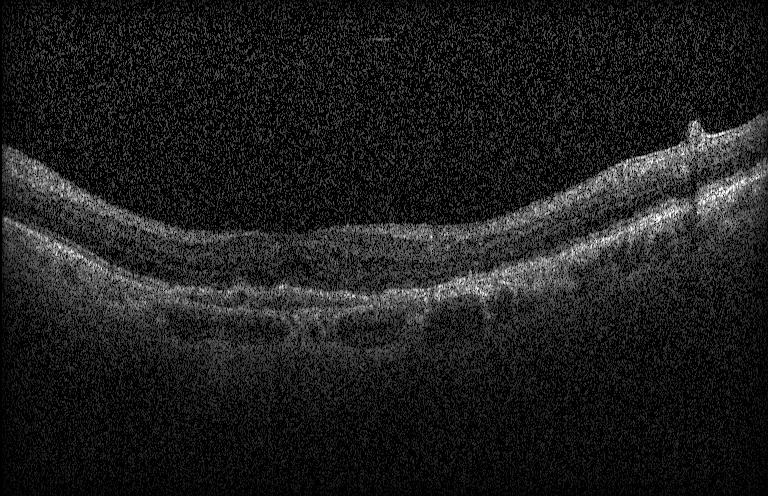 Macular OCT demonstrating choroidal neovascularization (CNV).